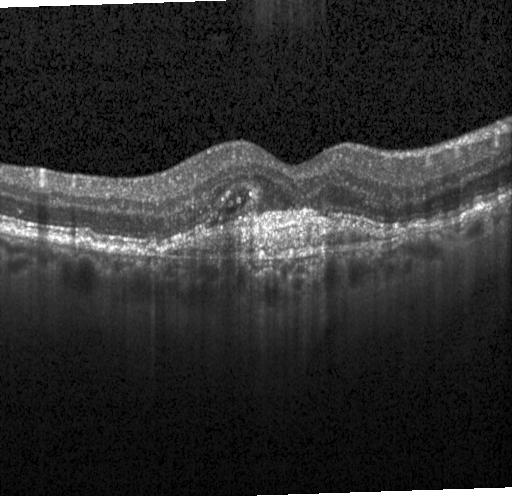 Centered on the fovea; Heidelberg Spectralis; retinal OCT cross-section.
Diagnosis: choroidal neovascularization.